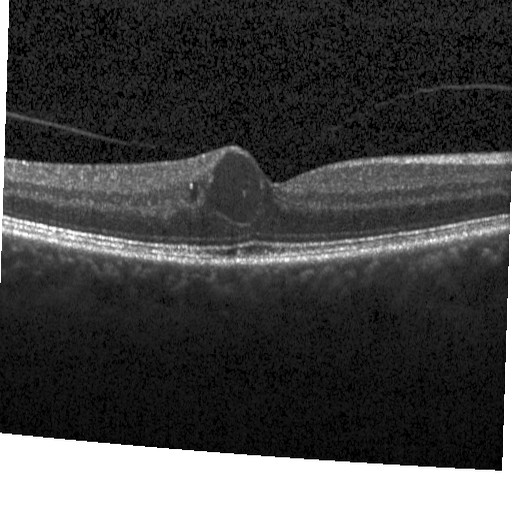

DME.